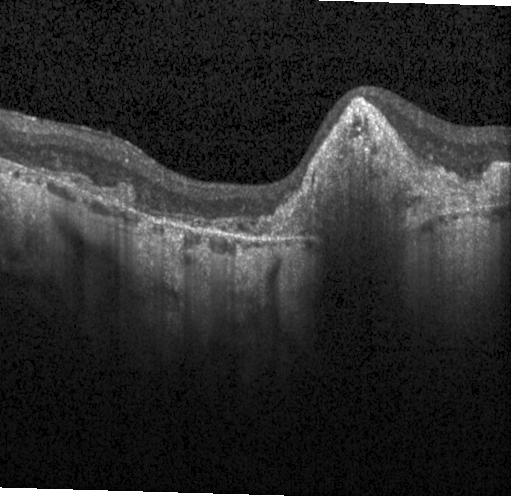

OCT finding: choroidal neovascularization (CNV).